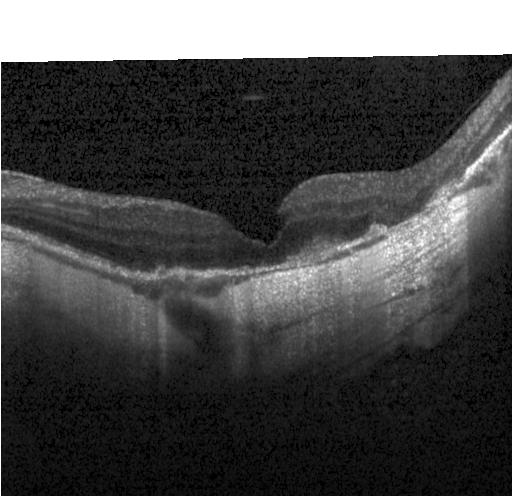
Fovea-centered · instrument: Heidelberg Spectralis · optical coherence tomography B-scan · SD-OCT.
This B-scan demonstrates a choroidal neovascular membrane.